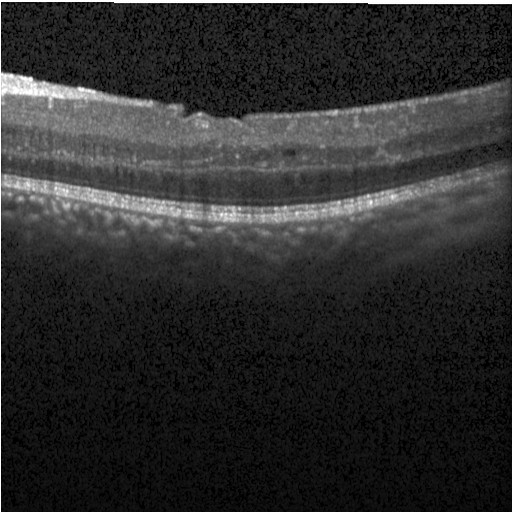

Horizontal scan through the fovea · retinal OCT B-scan · spectral-domain OCT · instrument: Heidelberg Spectralis
The scan shows diabetic macular edema (DME).